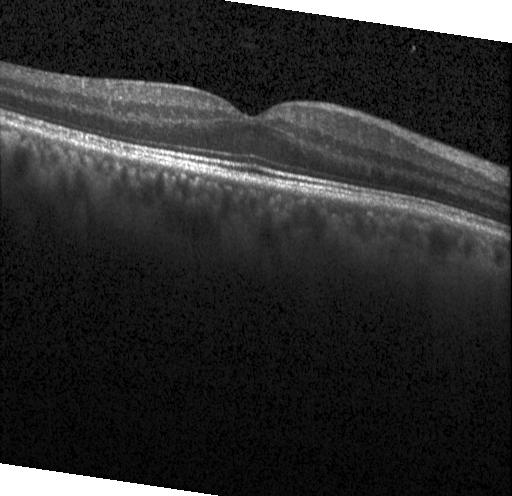

OCT line scan, through the macula, Heidelberg Spectralis.
This B-scan demonstrates no evidence of CNV, DME, or drusen.